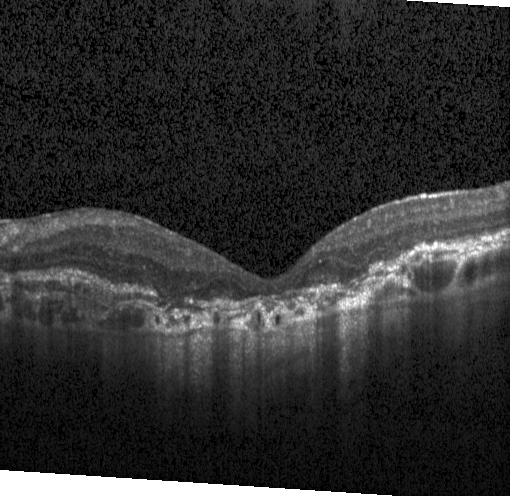 Centered on the fovea; acquired on a Heidelberg Spectralis; OCT B-scan. Macular OCT: a choroidal neovascular membrane.